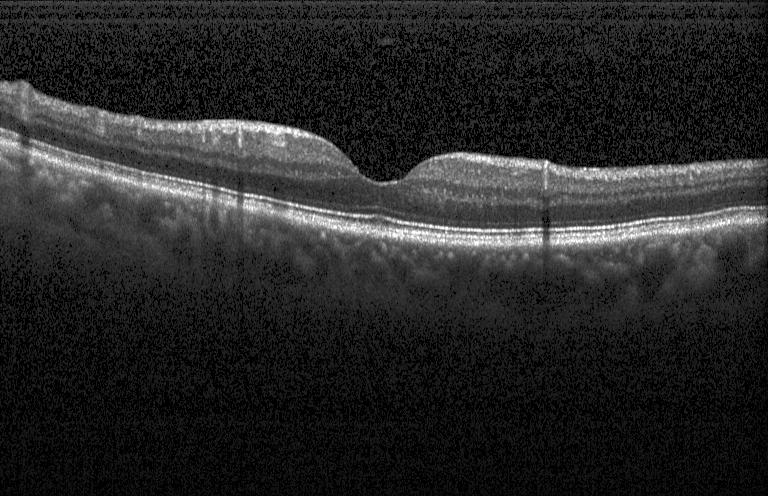
Optical coherence tomography scan. Impression: no CNV, no DME, and no drusen.